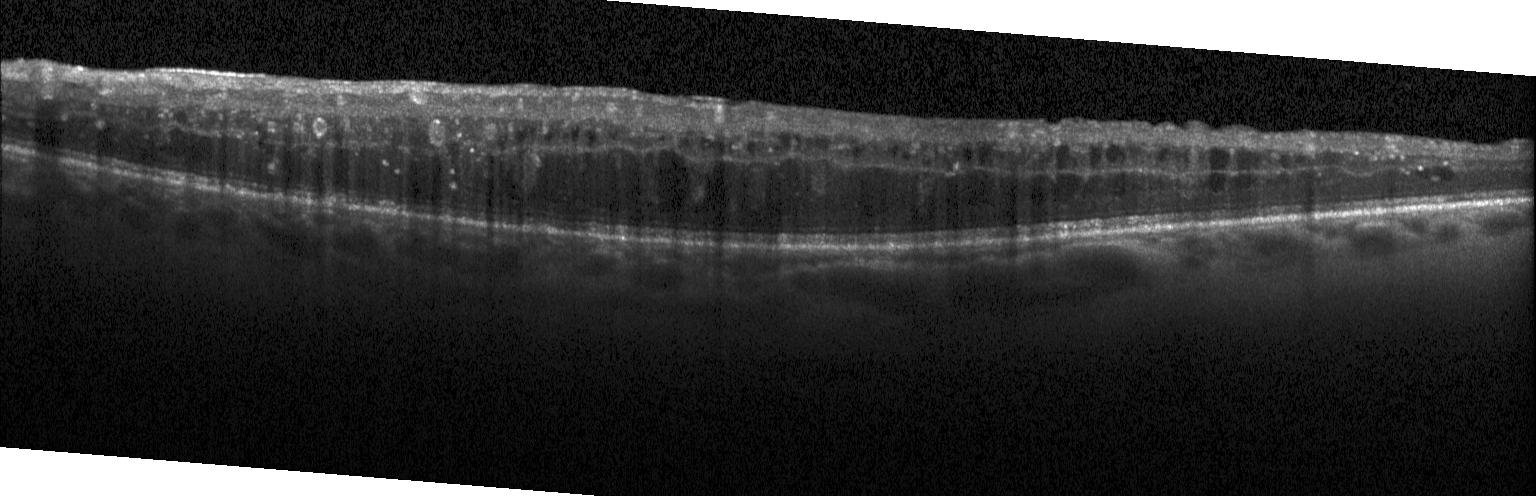

Optical coherence tomography scan; spectral-domain optical coherence tomography; fovea-centered; Heidelberg Spectralis — Diabetic macular edema.